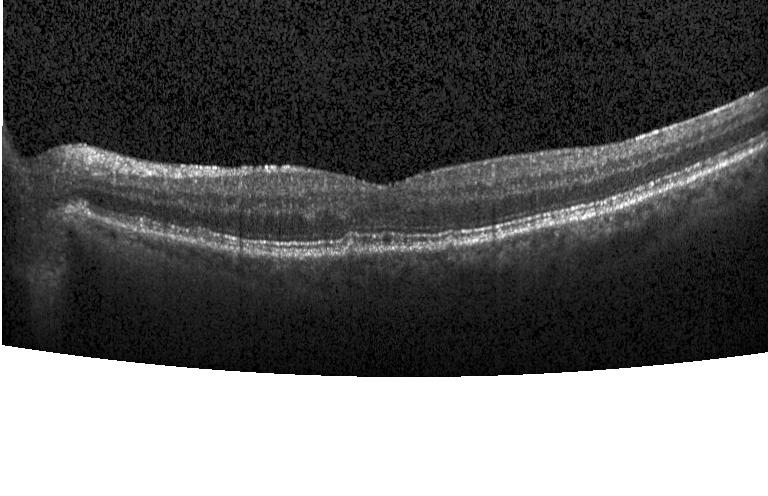 This B-scan demonstrates sub-RPE drusenoid deposits.